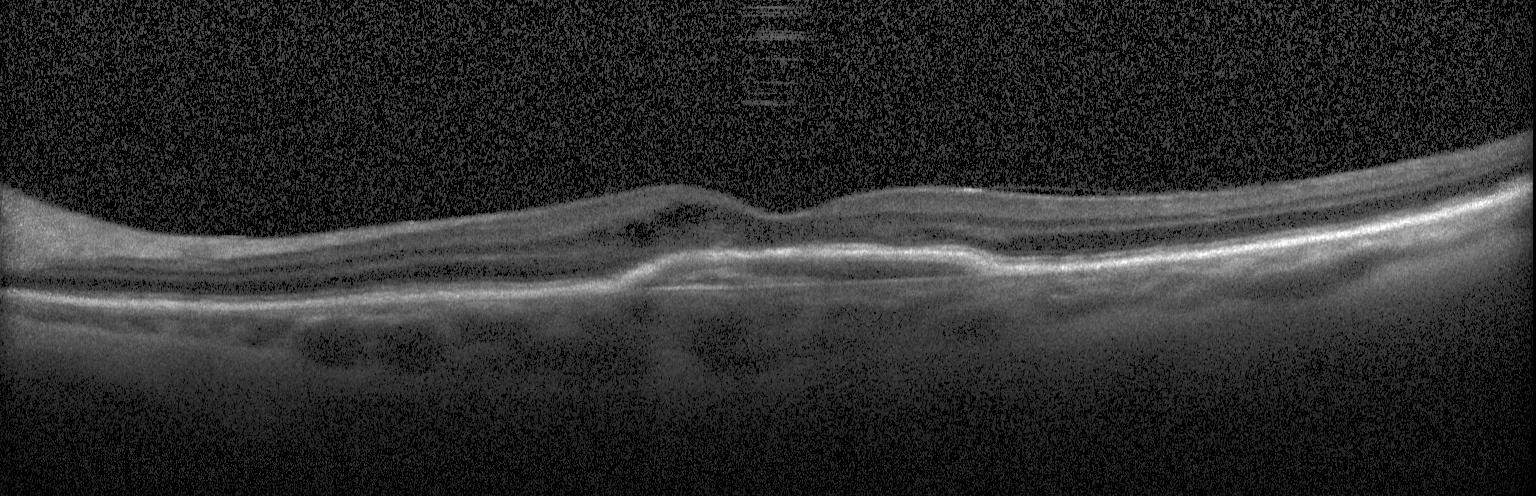

Optical coherence tomography B-scan — Finding: choroidal neovascularization (CNV).